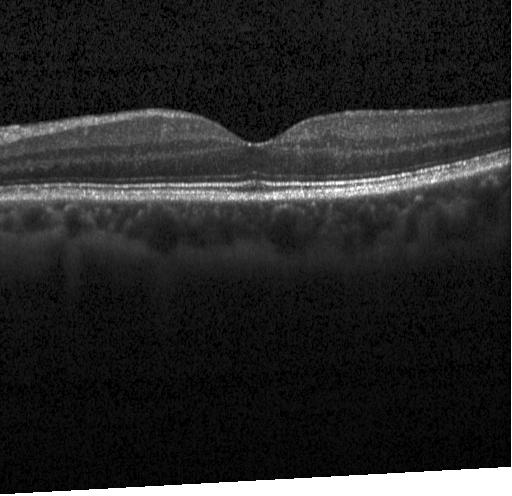
Diagnosis: no choroidal neovascularization, no diabetic macular edema, and no drusen.